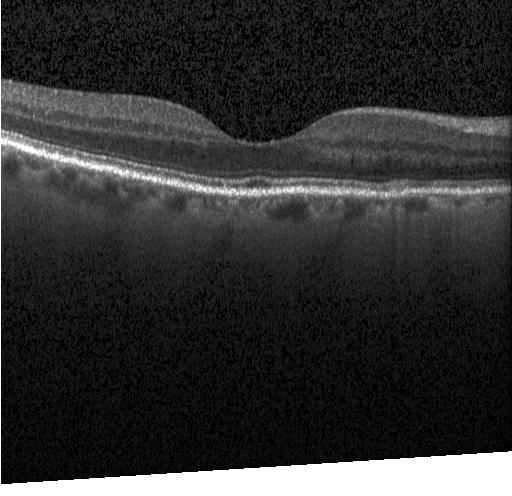 Retinal OCT cross-section showing no choroidal neovascularization, diabetic macular edema, or drusen.